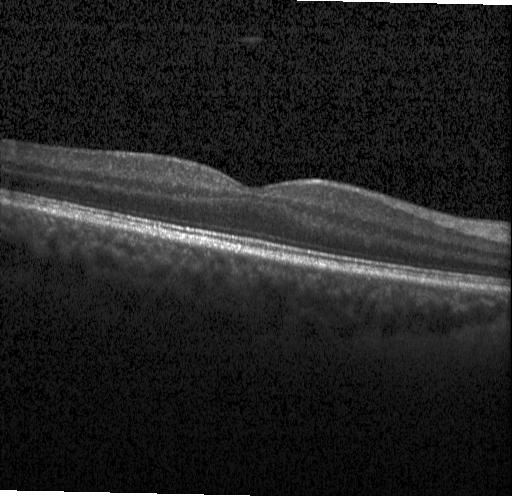 Heidelberg Spectralis. Horizontal scan through the fovea. Optical coherence tomography scan. Impression: neither choroidal neovascularization, diabetic macular edema, nor drusen.